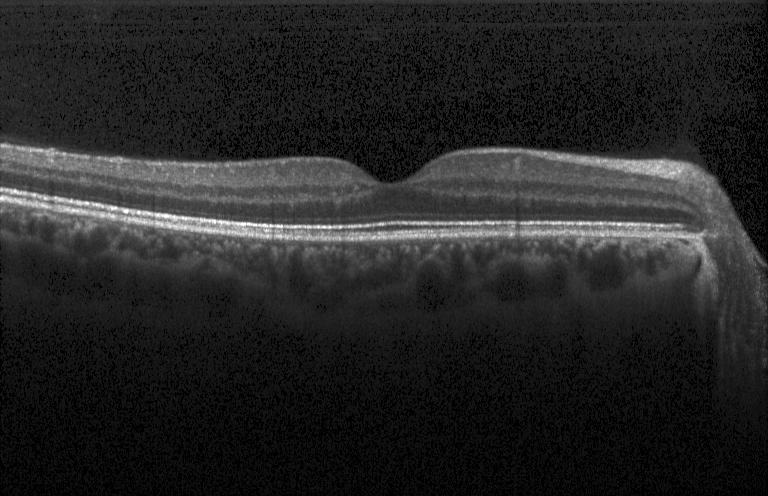

Impression: no choroidal neovascularization, diabetic macular edema, or drusen.